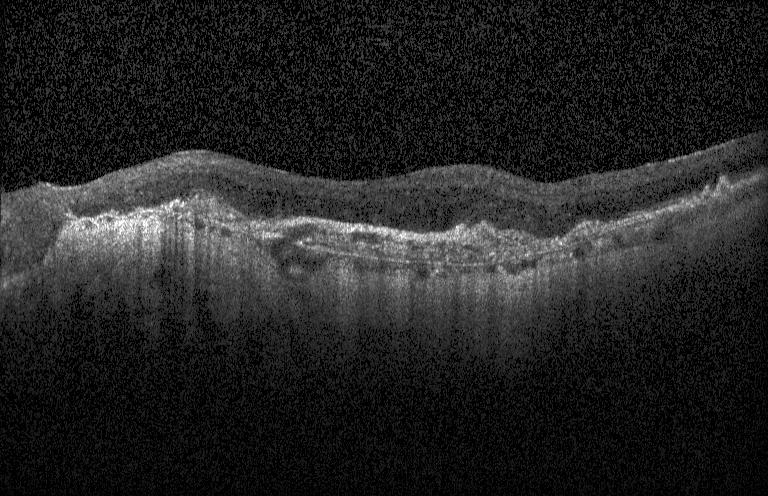

This B-scan demonstrates choroidal neovascularization (CNV).